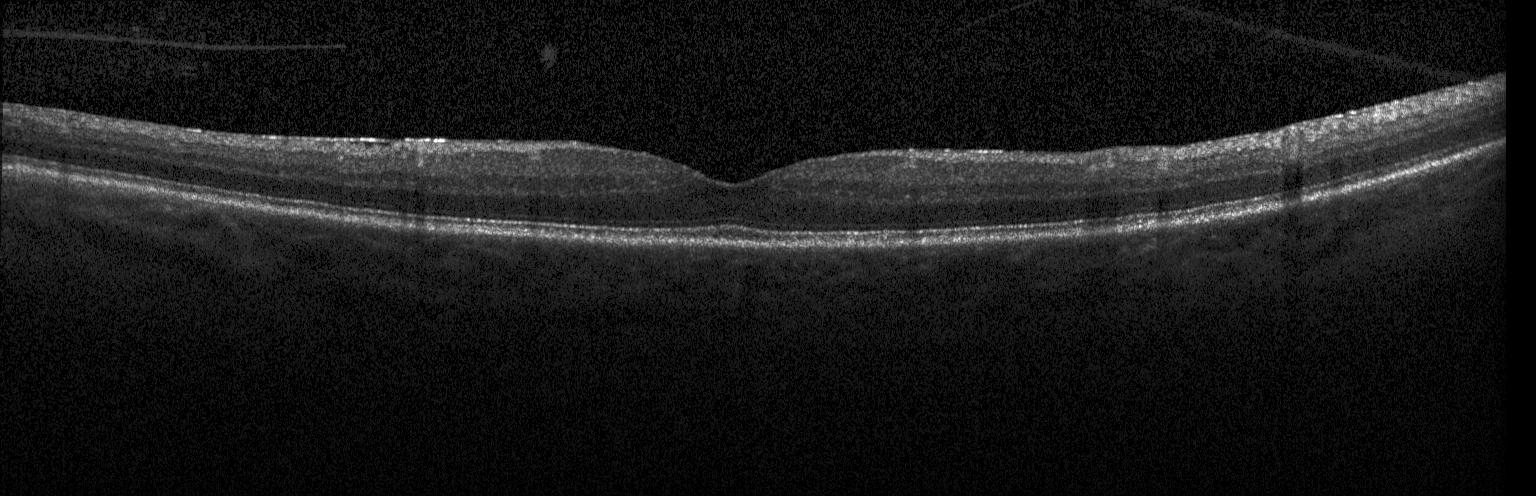

SD-OCT; instrument: Heidelberg Spectralis; fovea-centered; optical coherence tomography scan
Diagnosis: neither choroidal neovascularization, diabetic macular edema, nor drusen.